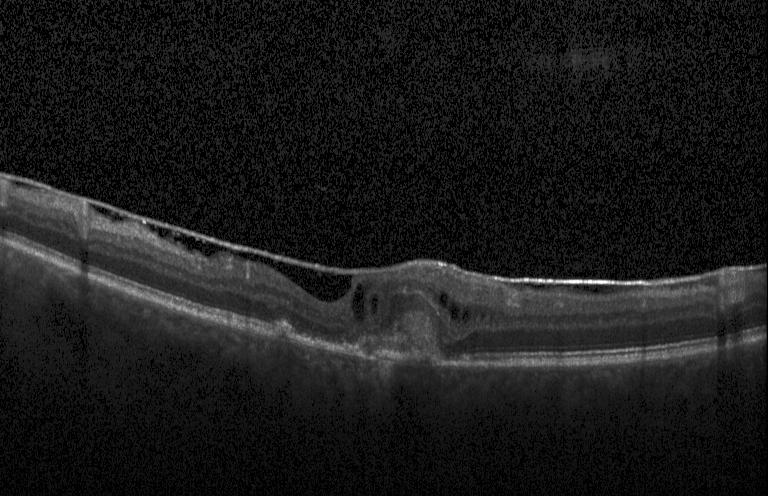

OCT line scan; Heidelberg Spectralis — This B-scan demonstrates CNV.